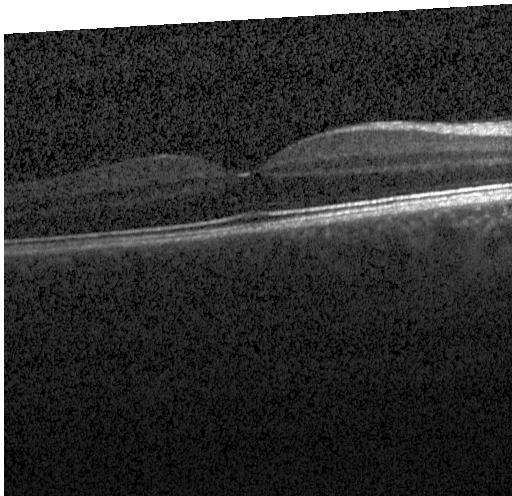
Optical coherence tomography B-scan.
Dx: neither choroidal neovascularization, diabetic macular edema, nor drusen.